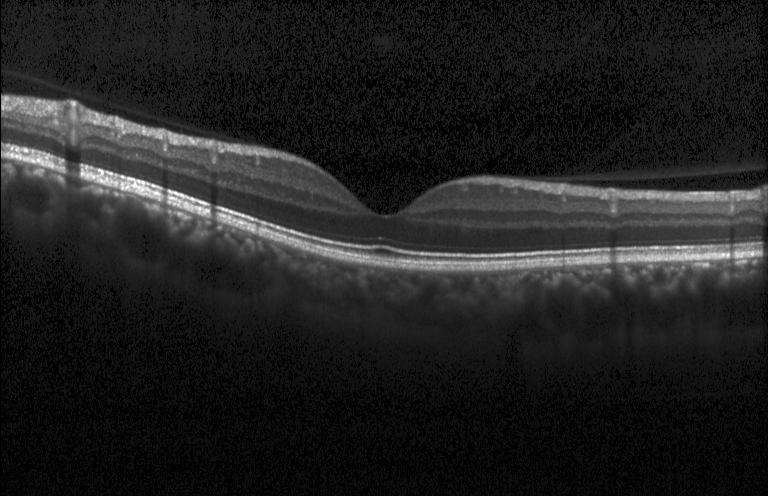
Optical coherence tomography B-scan; spectral-domain optical coherence tomography; acquired on a Heidelberg Spectralis.
Diagnosis: neither CNV, DME, nor drusen.